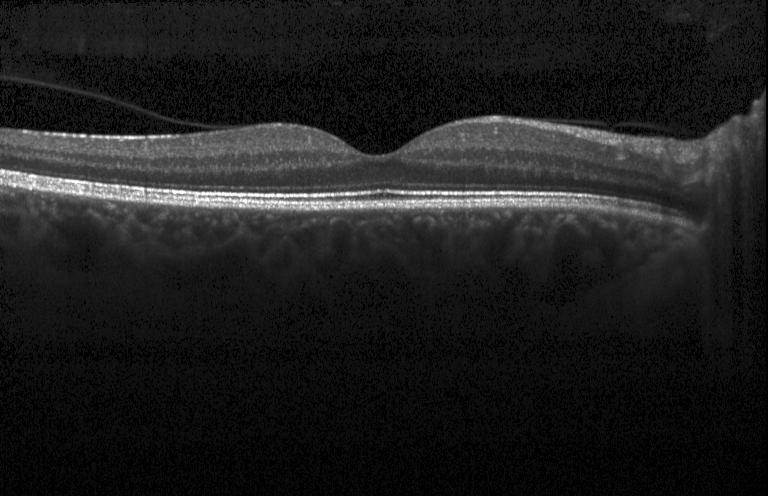

Retinal OCT cross-section.
The scan shows no choroidal neovascularization, diabetic macular edema, or drusen.